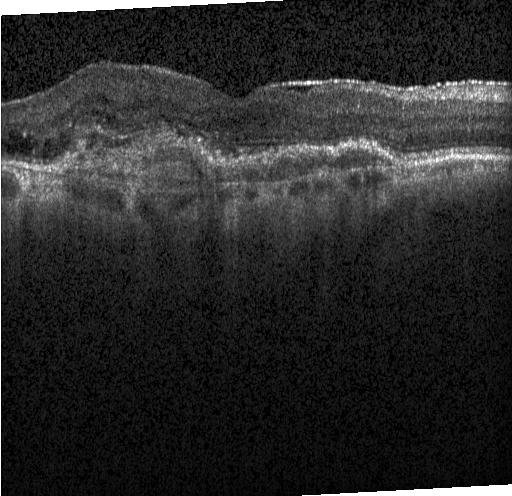

Retinal OCT B-scan
This B-scan demonstrates CNV.